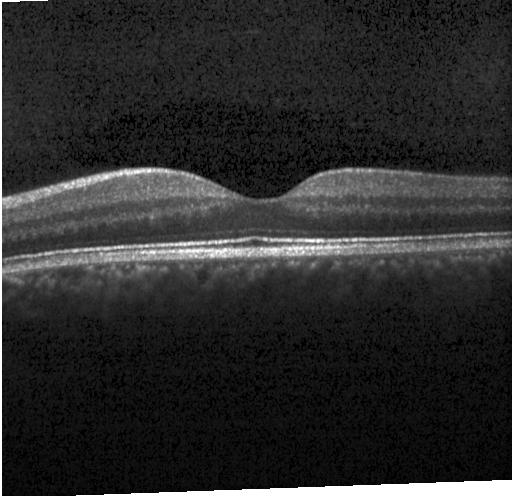

Retinal OCT cross-section
Diagnosis: no CNV, DME, or drusen.